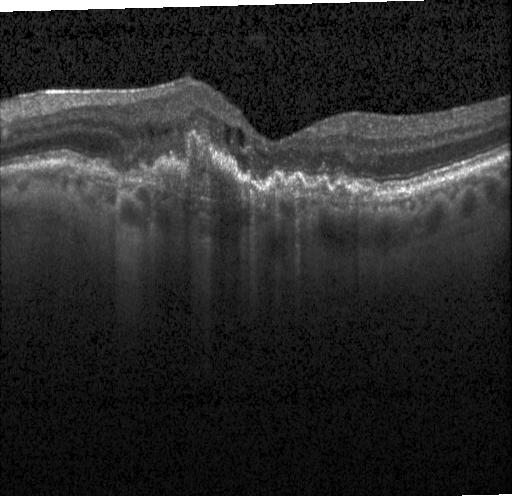

Through the macula · OCT line scan · Heidelberg Spectralis OCT system · spectral-domain optical coherence tomography.
Macular OCT: a choroidal neovascular membrane.